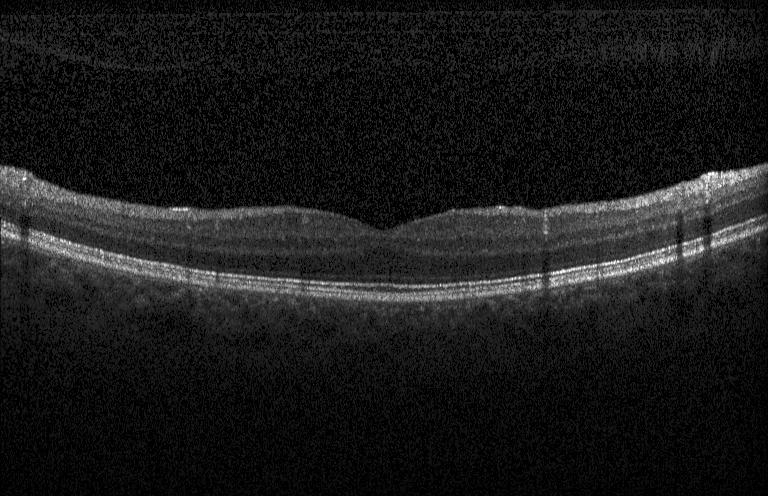
Finding: neither choroidal neovascularization, diabetic macular edema, nor drusen.